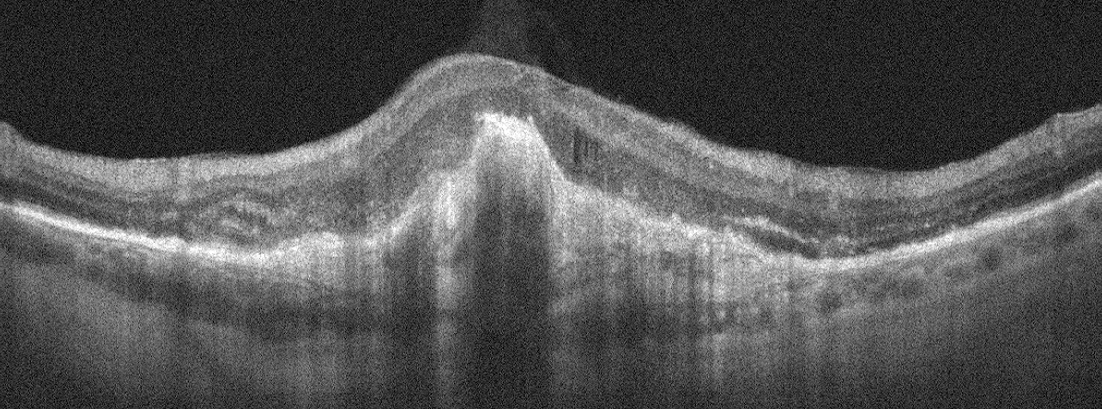

Optical coherence tomography B-scan
Macular OCT: age-related macular degeneration.